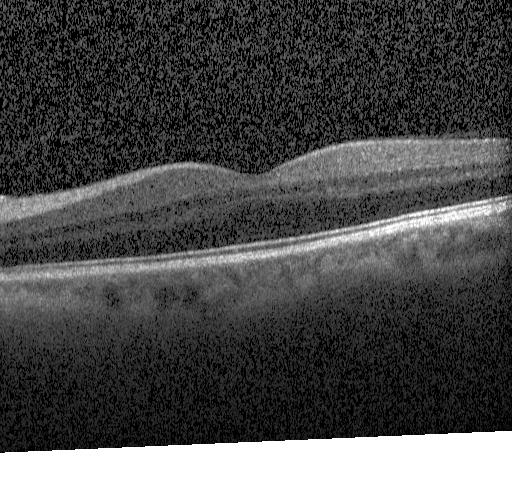 Spectral-domain optical coherence tomography, instrument: Heidelberg Spectralis, OCT B-scan. The scan shows no CNV, no DME, and no drusen.